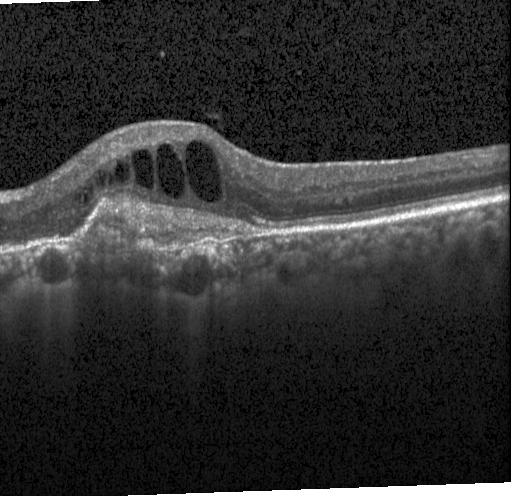

Optical coherence tomography scan. Spectral-domain optical coherence tomography. Heidelberg Spectralis.
Assessment: a choroidal neovascular membrane.